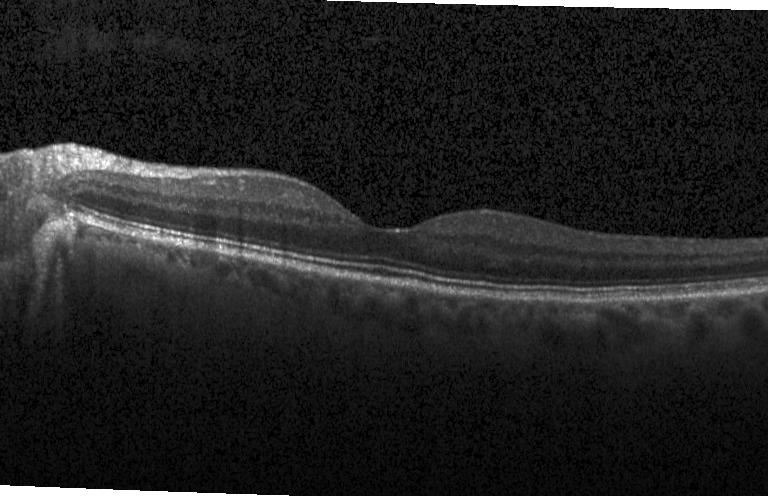

Through the macula; retinal OCT B-scan; spectral-domain optical coherence tomography; Heidelberg Spectralis.
This B-scan demonstrates no choroidal neovascularization, no diabetic macular edema, and no drusen.